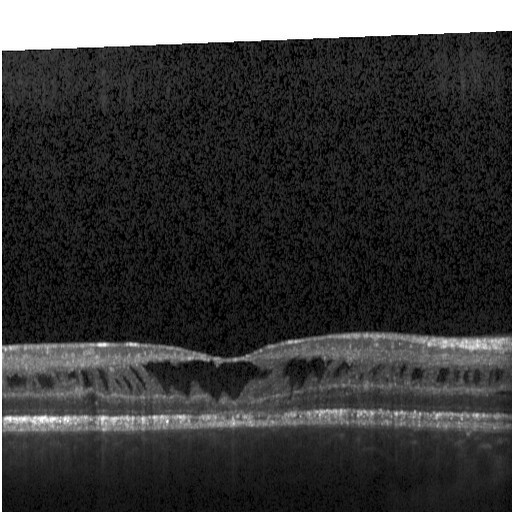 Macular scan · SD-OCT · instrument: Heidelberg Spectralis · retinal OCT cross-section. Diagnosis: diabetic macular edema.